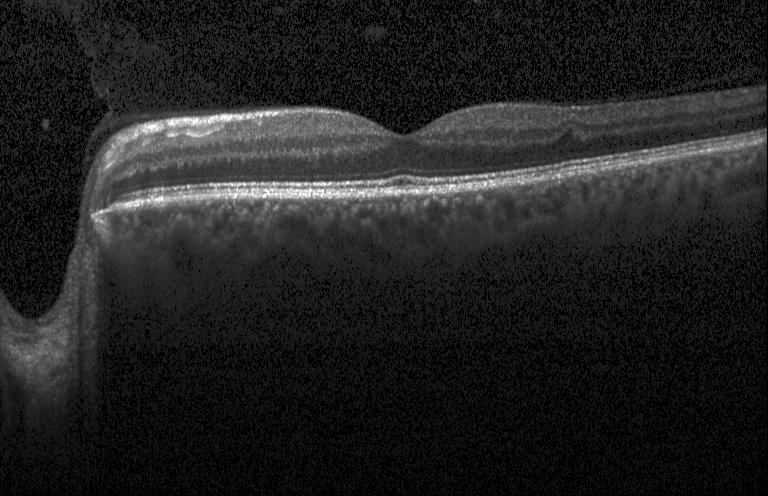

SD-OCT. Optical coherence tomography scan. Neither choroidal neovascularization, diabetic macular edema, nor drusen.